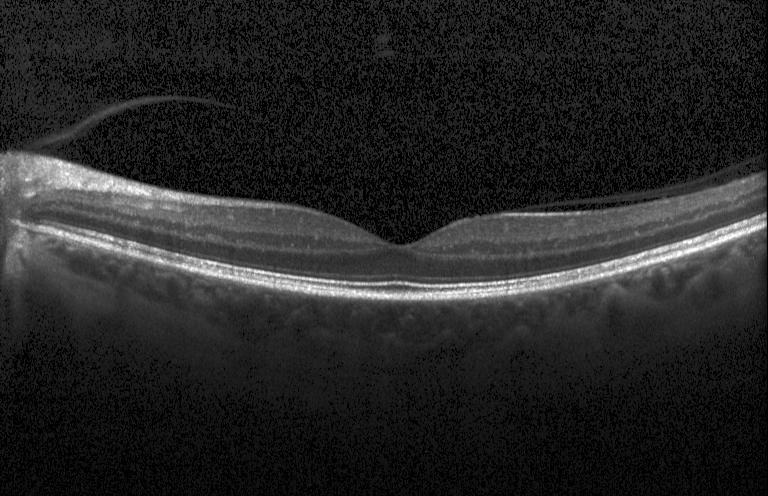
OCT B-scan. Finding: no choroidal neovascularization, diabetic macular edema, or drusen.